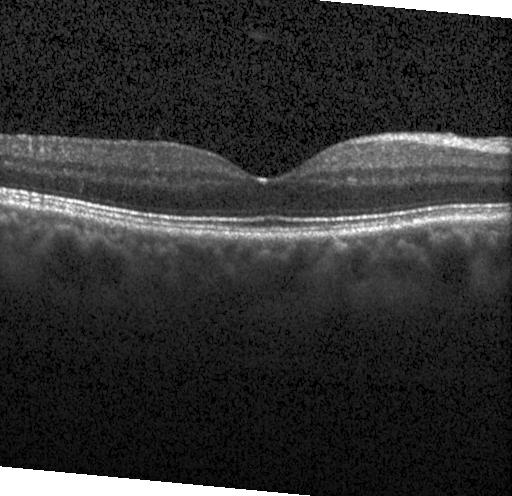

Instrument: Heidelberg Spectralis · fovea-centered · OCT B-scan.
Diagnosis: no evidence of choroidal neovascularization, diabetic macular edema, or drusen.